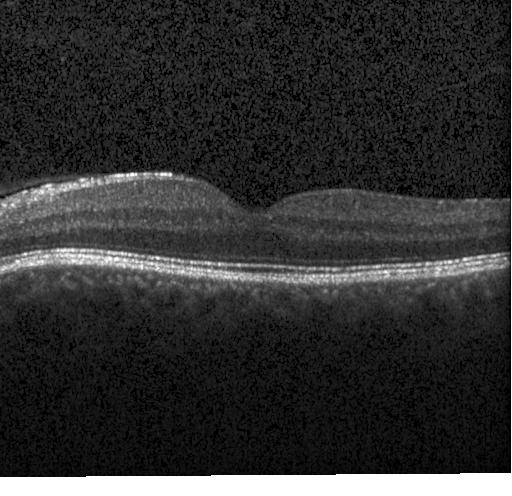

Acquired on a Heidelberg Spectralis; optical coherence tomography scan. Diagnosis: no evidence of choroidal neovascularization, diabetic macular edema, or drusen.